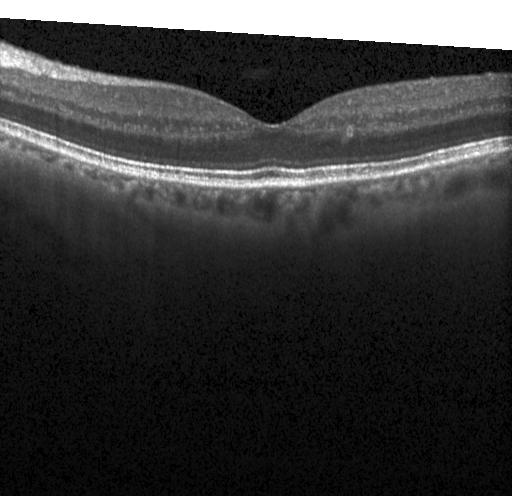

Through the macula · OCT B-scan — No CNV, DME, or drusen.